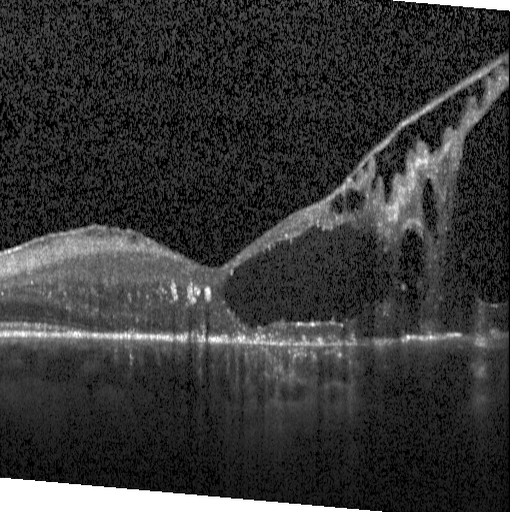 Optical coherence tomography B-scan.
Diagnosis: diabetic macular edema (DME).